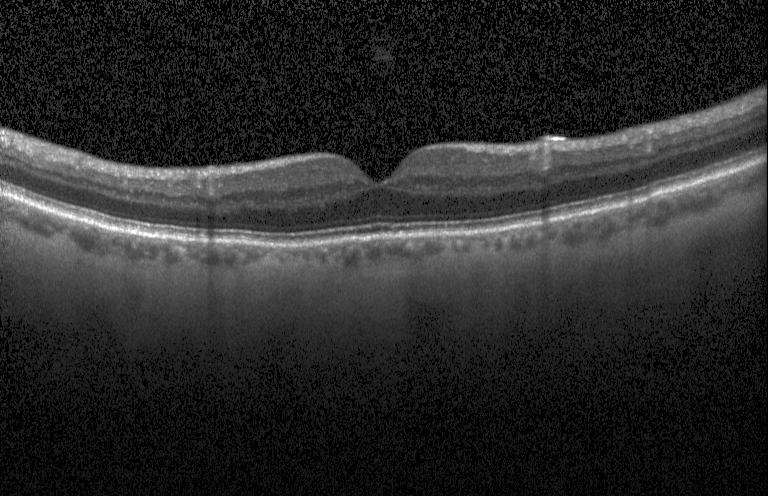 OCT finding: no evidence of choroidal neovascularization, diabetic macular edema, or drusen.